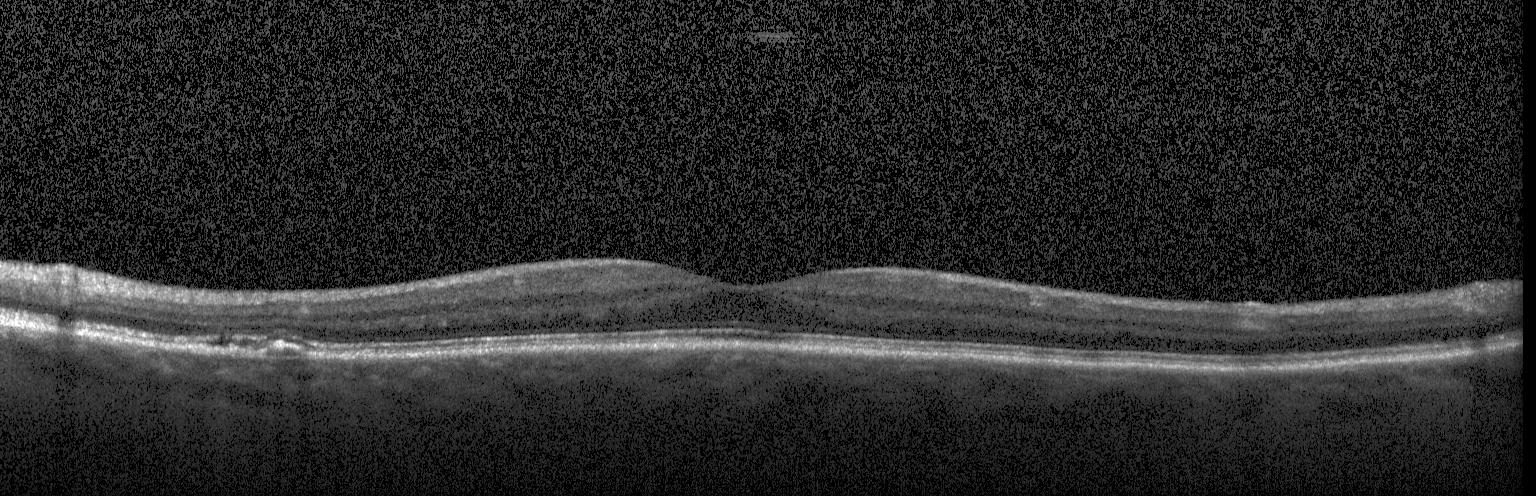

OCT B-scan.
Assessment: a choroidal neovascular membrane.